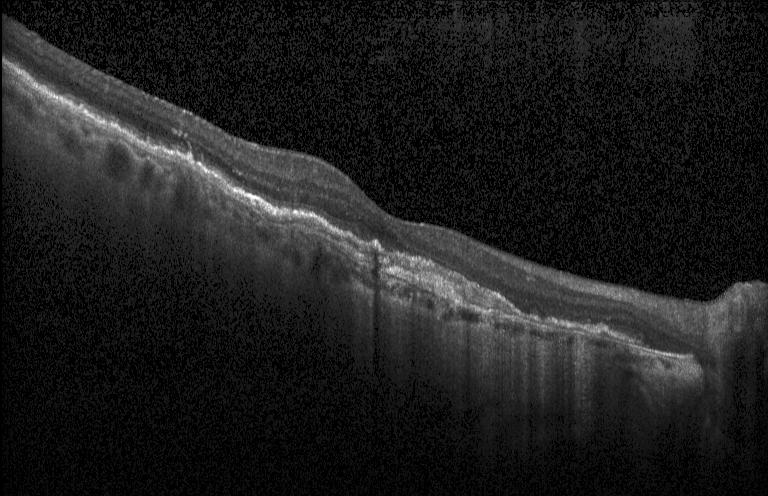 OCT B-scan.
Diagnosis: a choroidal neovascular membrane.